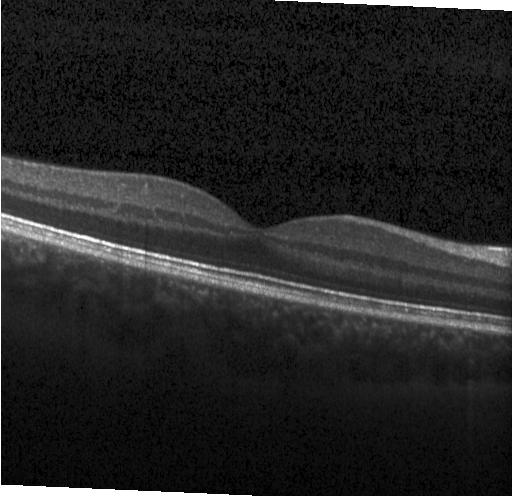
Instrument: Heidelberg Spectralis. Spectral-domain optical coherence tomography. Retinal OCT cross-section. Macular scan. The scan shows neither choroidal neovascularization, diabetic macular edema, nor drusen.